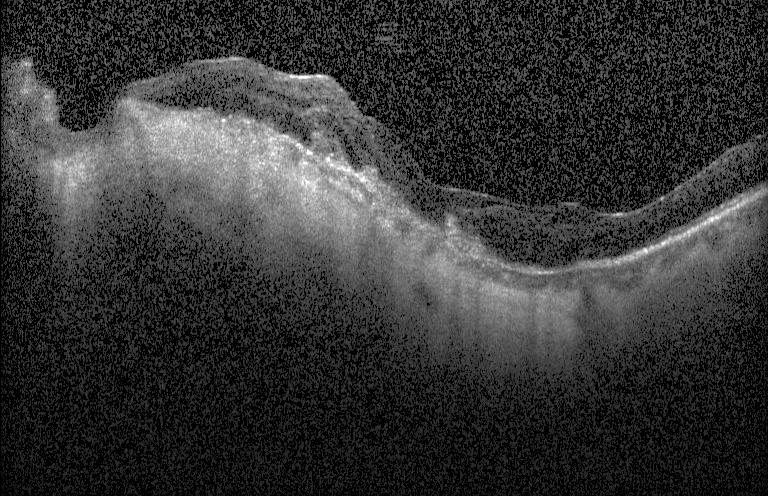
OCT finding: a choroidal neovascular membrane.